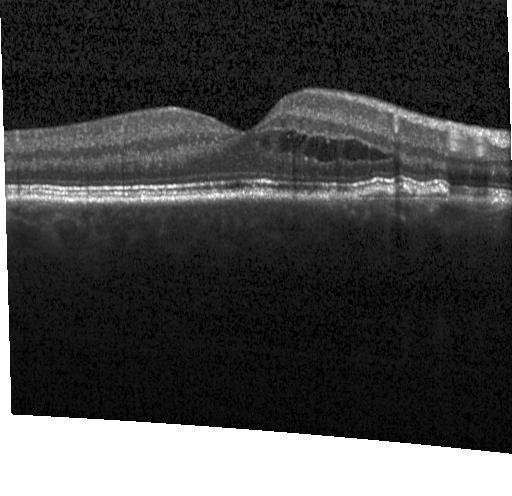

Macular OCT demonstrating choroidal neovascularization.